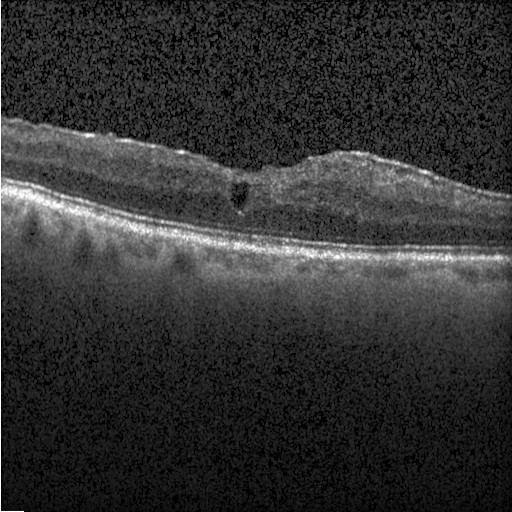

Acquired on a Heidelberg Spectralis, through the macula, retinal OCT cross-section
Diabetic macular edema.